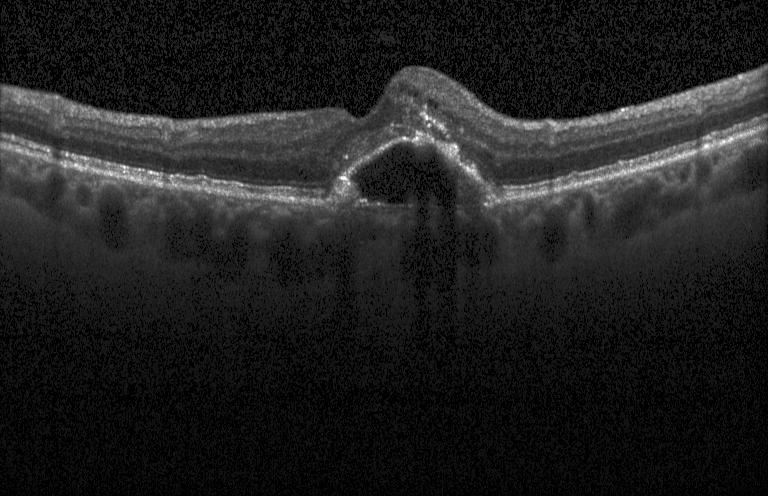

Acquired on a Heidelberg Spectralis, retinal OCT cross-section. Impression: a choroidal neovascular membrane.